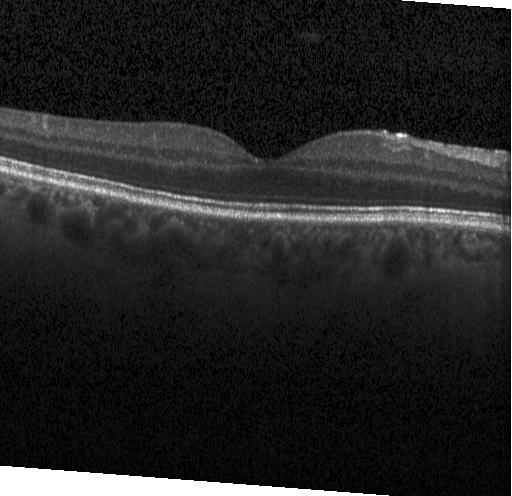
Horizontal scan through the fovea, optical coherence tomography B-scan, spectral-domain OCT — Impression: no choroidal neovascularization, diabetic macular edema, or drusen.